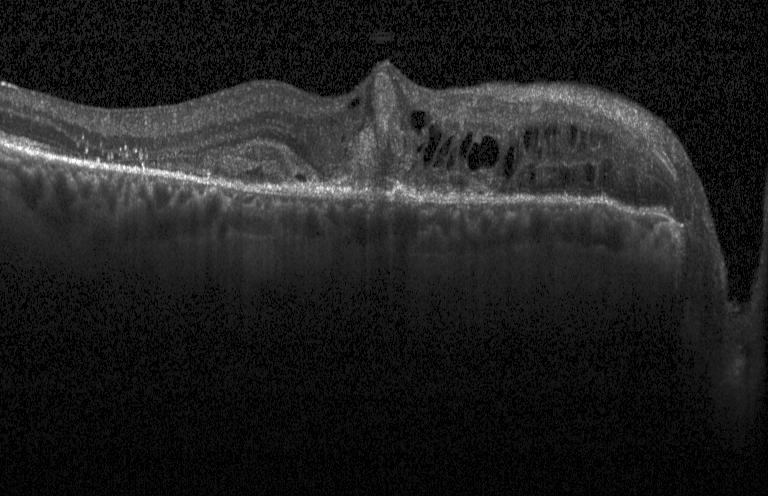

Retinal OCT cross-section showing a choroidal neovascular membrane.